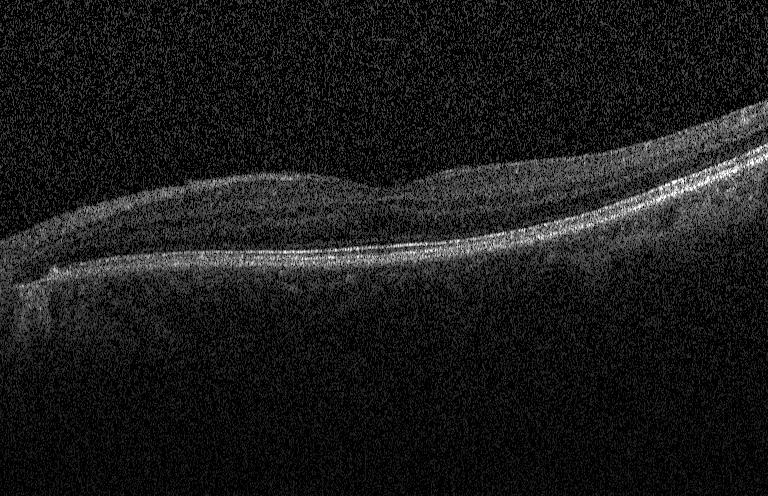

Impression: neither choroidal neovascularization, diabetic macular edema, nor drusen.